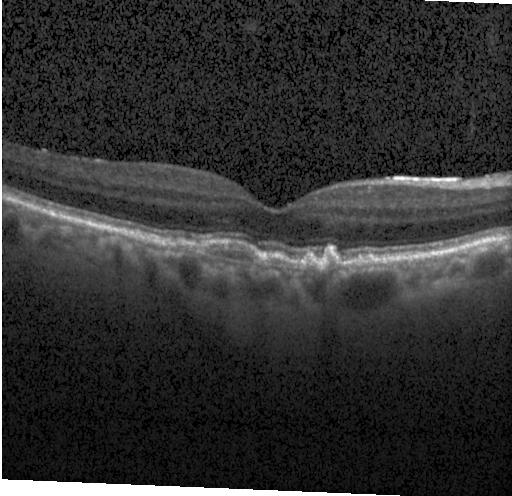
Impression: a choroidal neovascular membrane.